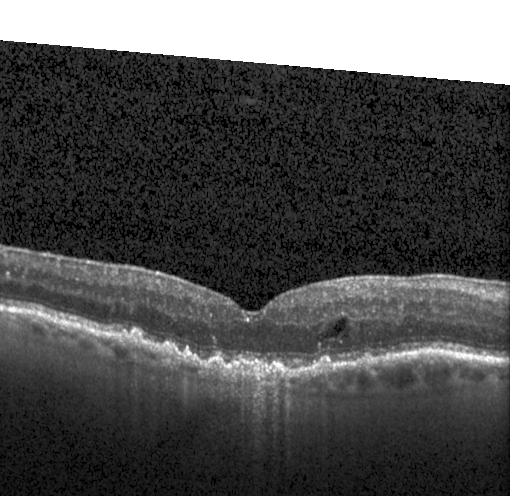
Macular OCT: a choroidal neovascular membrane.